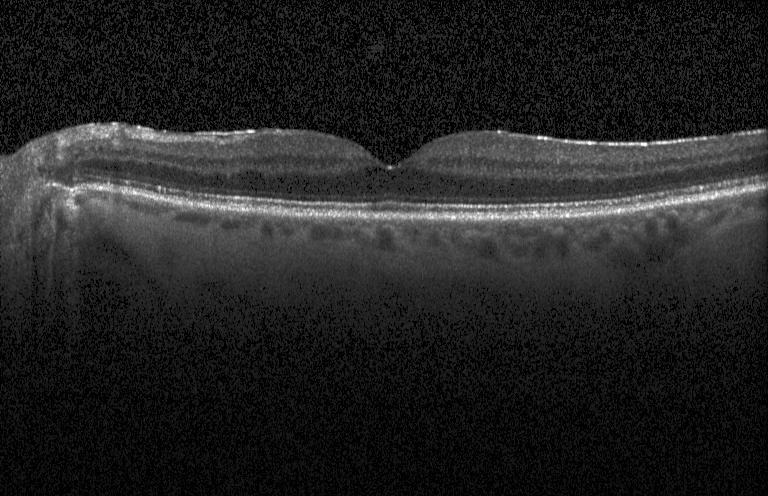

The scan shows no choroidal neovascularization, no diabetic macular edema, and no drusen.